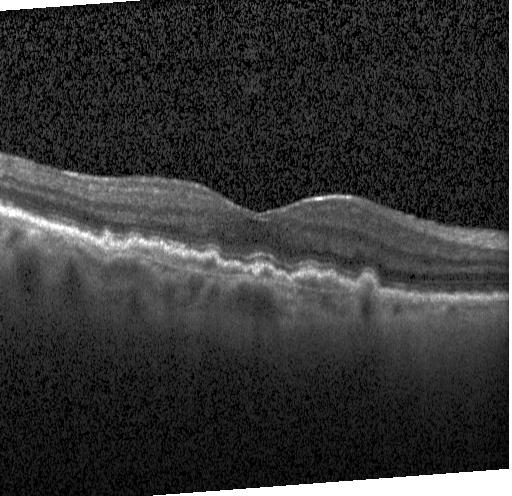
Optical coherence tomography scan; through the macula; Heidelberg Spectralis OCT system; spectral-domain OCT — Diagnosis: CNV.